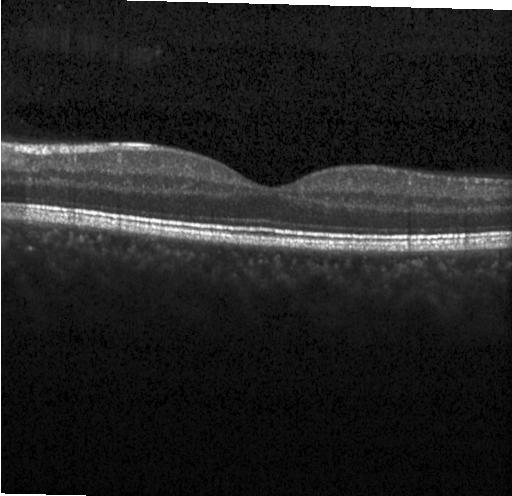

OCT finding: no CNV, DME, or drusen.